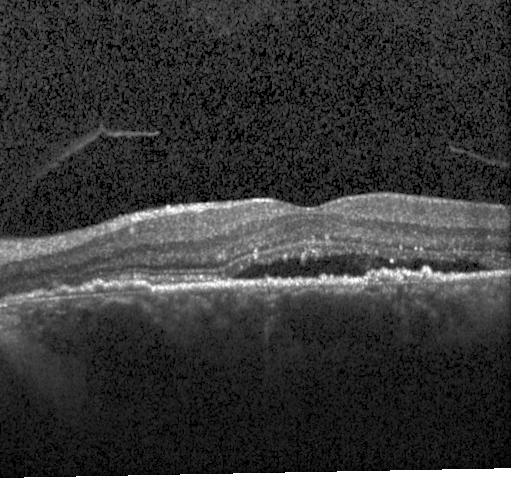 Fovea-centered; OCT line scan; acquired on a Heidelberg Spectralis; SD-OCT
This B-scan demonstrates a choroidal neovascular membrane.